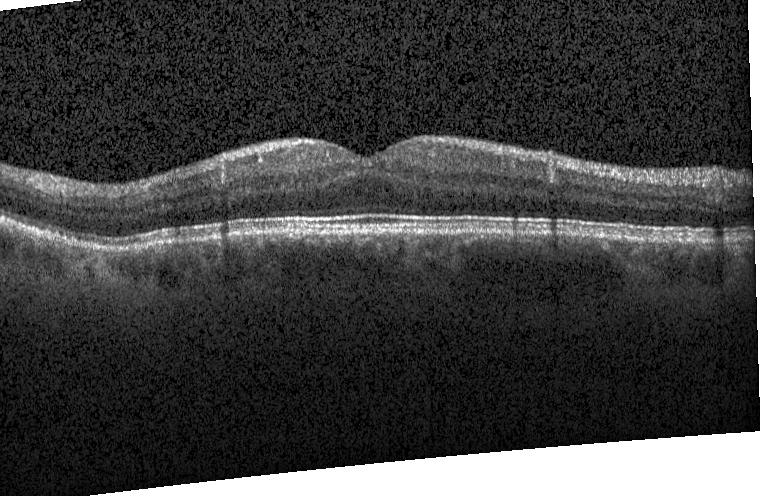
Retinal OCT cross-section, Heidelberg Spectralis OCT system — Impression: no choroidal neovascularization, diabetic macular edema, or drusen.